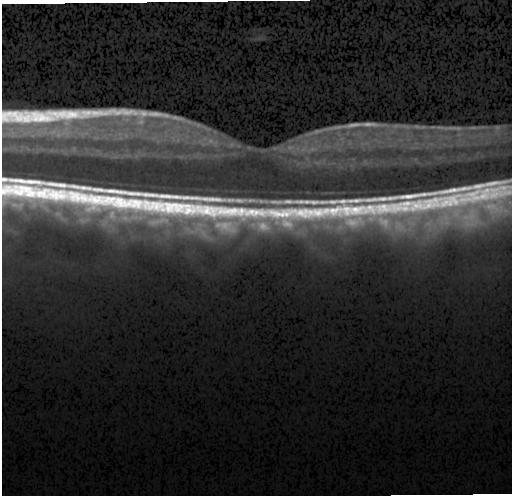 No evidence of choroidal neovascularization, diabetic macular edema, or drusen.